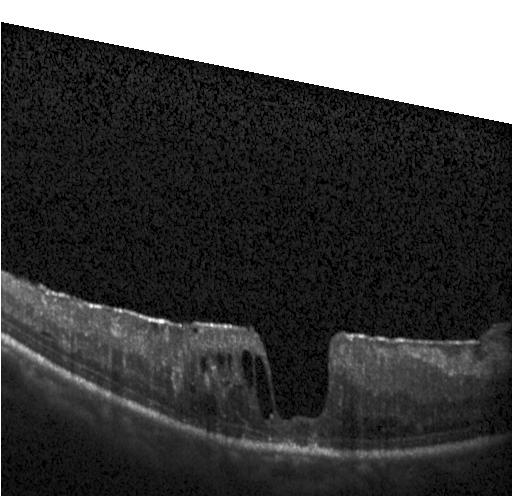

Diagnosis: diabetic macular edema.